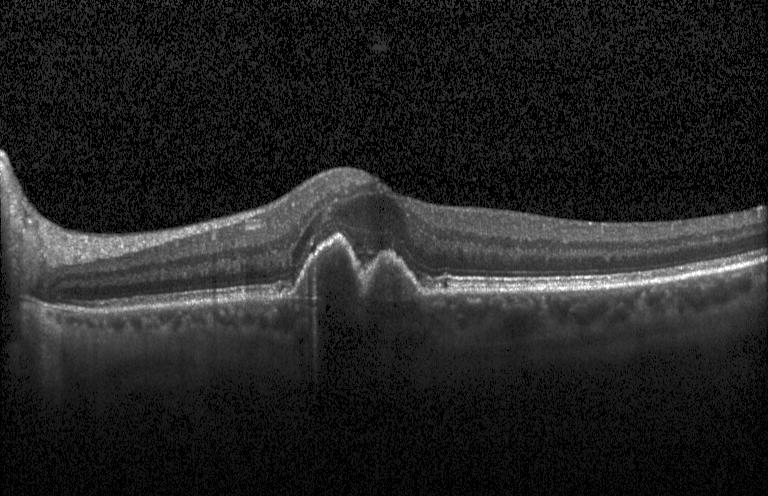 Retinal OCT B-scan — Impression: CNV.